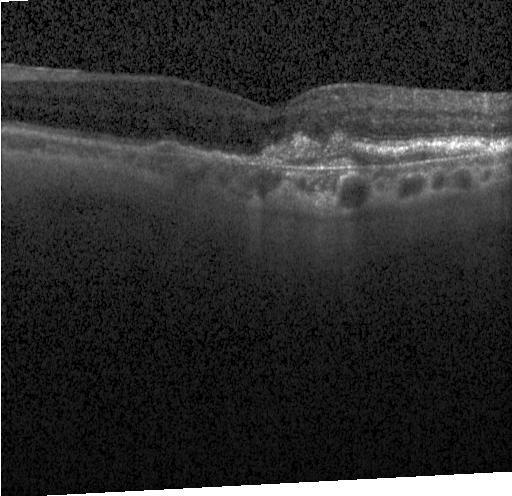
Centered on the fovea · Heidelberg Spectralis OCT system · retinal OCT cross-section — Impression: choroidal neovascularization (CNV).